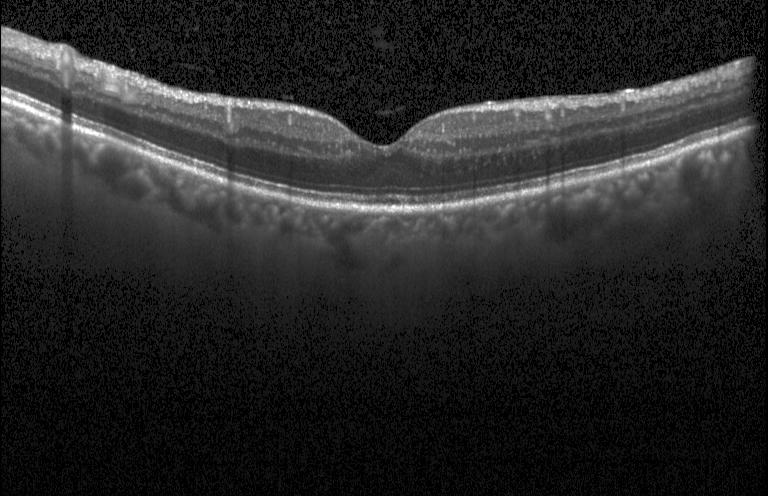

Retinal OCT cross-section showing no choroidal neovascularization, no diabetic macular edema, and no drusen.